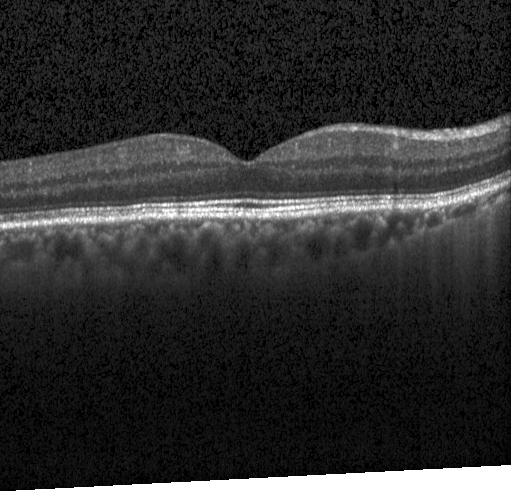

OCT scan showing neither CNV, DME, nor drusen.